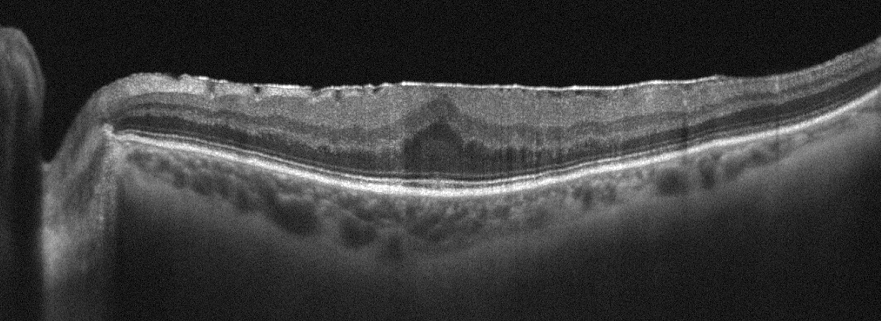

Acquired on an Optovue Avanti RTVue XR. Fovea-centered. Retinal OCT cross-section — ERM.